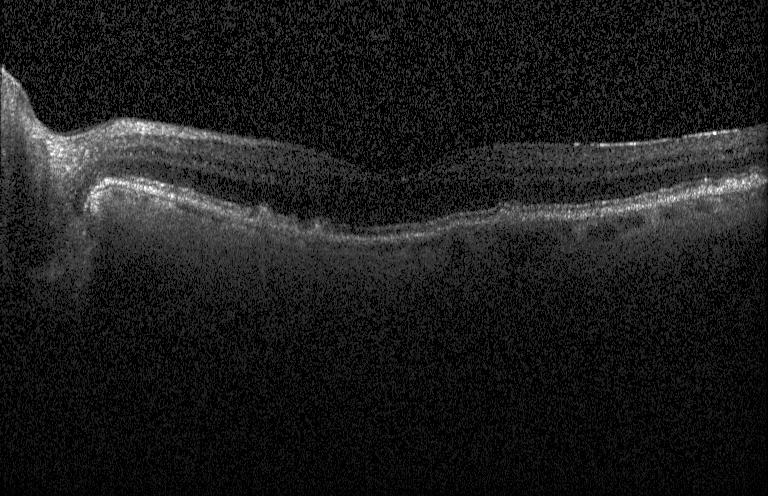 Finding: multiple drusen.